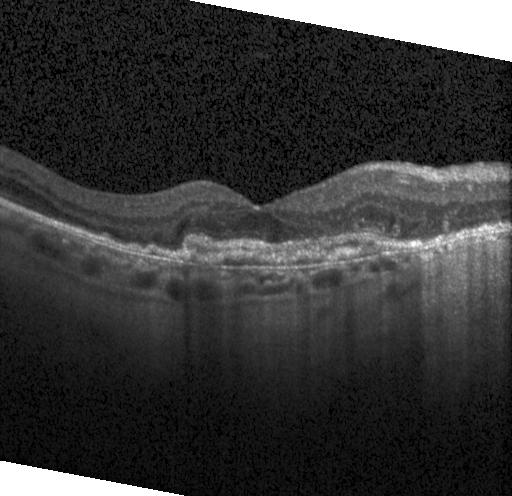 Optical coherence tomography B-scan.
Diagnosis: choroidal neovascularization (CNV).